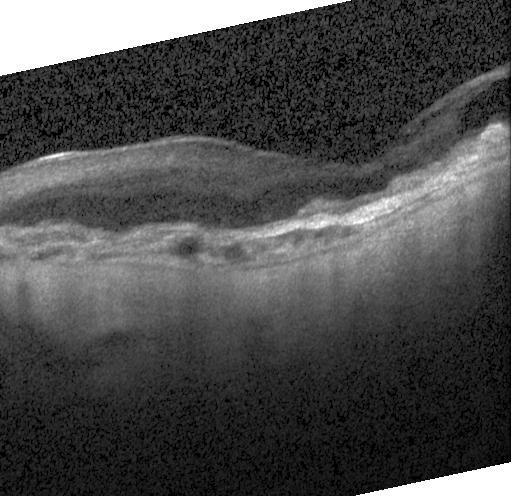
Dx: a choroidal neovascular membrane.